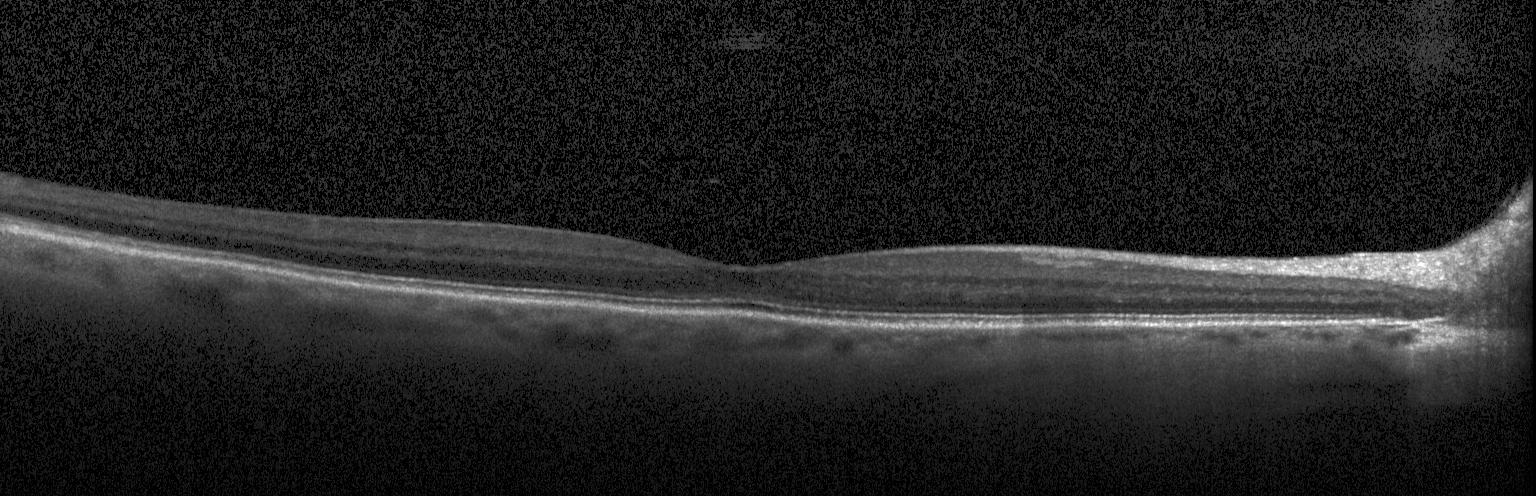
Macular OCT: no evidence of choroidal neovascularization, diabetic macular edema, or drusen.